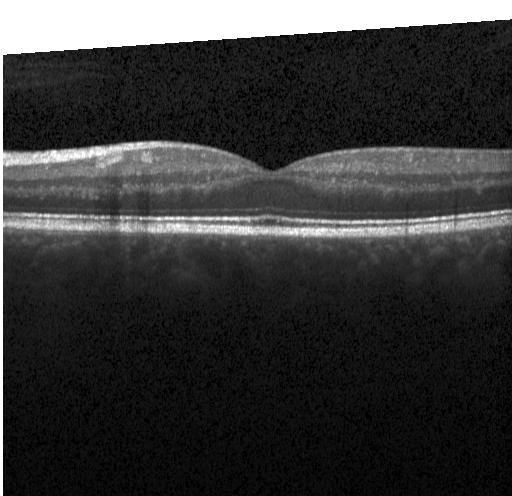
Optical coherence tomography B-scan.
Assessment: no evidence of CNV, DME, or drusen.